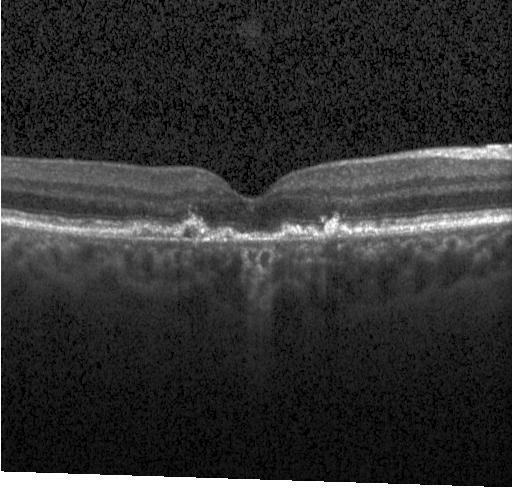 Impression: choroidal neovascularization.